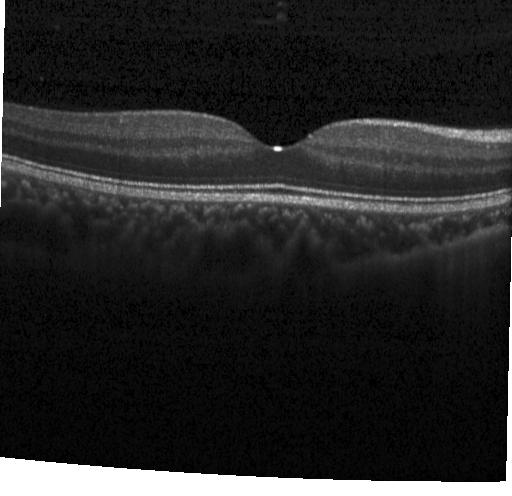

SD-OCT · OCT B-scan · through the macula.
Finding: no choroidal neovascularization, diabetic macular edema, or drusen.